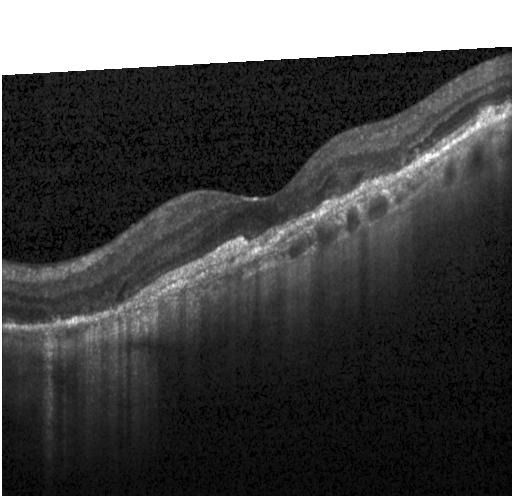

Acquired on a Heidelberg Spectralis, spectral-domain OCT, centered on the fovea, OCT line scan.
Impression: a choroidal neovascular membrane.